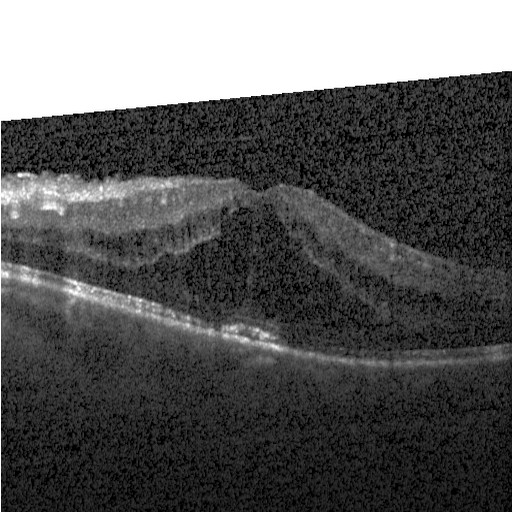

OCT line scan; Heidelberg Spectralis OCT system; SD-OCT. The scan shows diabetic macular edema (DME).